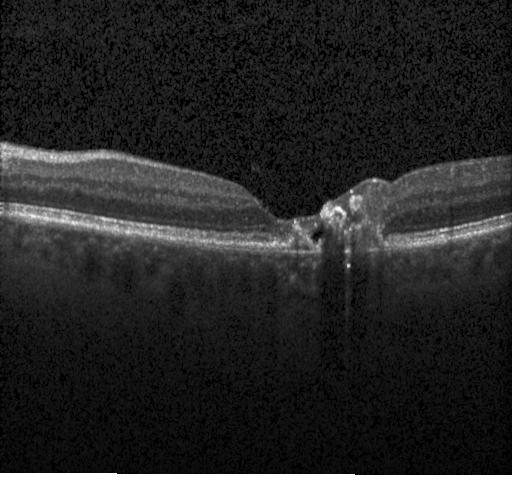 OCT B-scan. Spectral-domain optical coherence tomography.
This B-scan demonstrates a choroidal neovascular membrane.